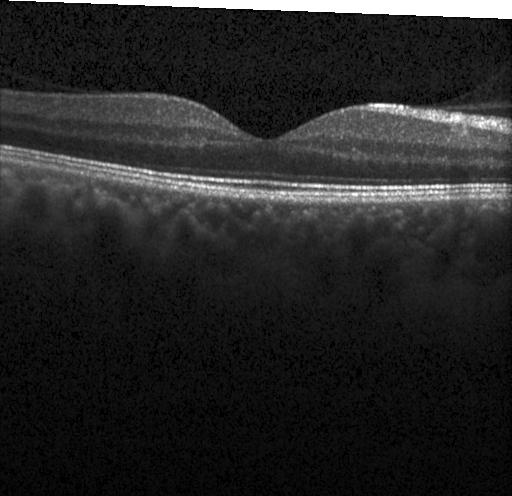

Heidelberg Spectralis OCT system, spectral-domain OCT, retinal OCT cross-section, horizontal scan through the fovea — This B-scan demonstrates no choroidal neovascularization, no diabetic macular edema, and no drusen.